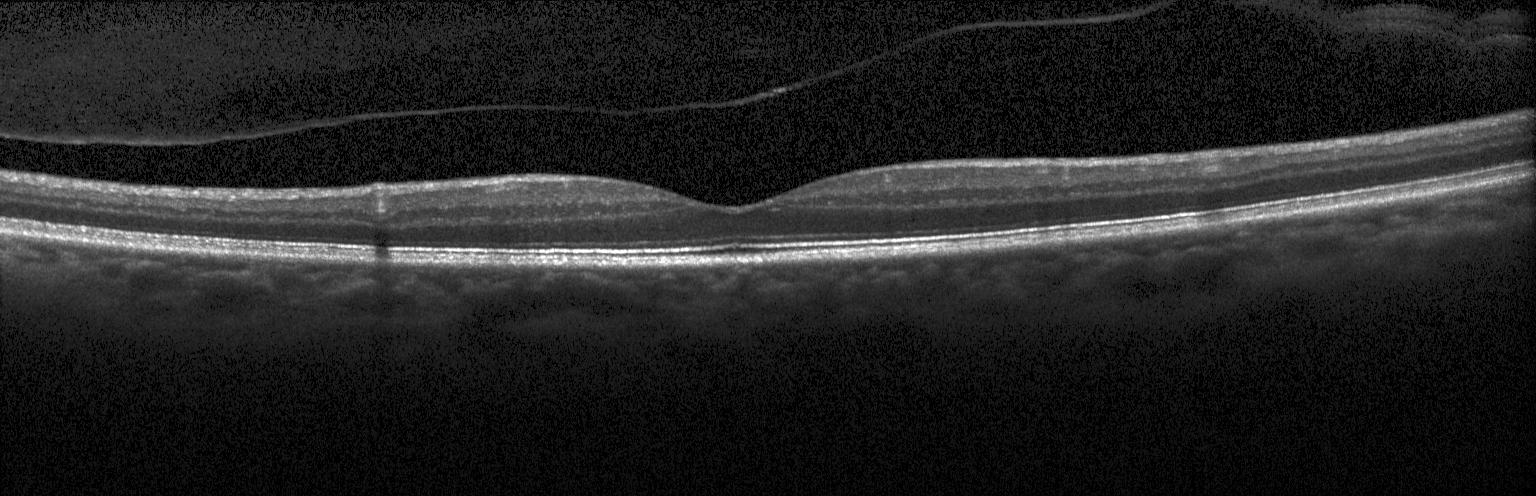
Macular OCT: no evidence of choroidal neovascularization, diabetic macular edema, or drusen.